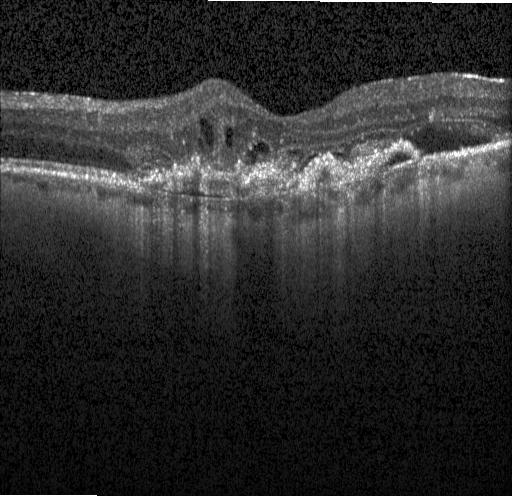
Macular scan, OCT B-scan, SD-OCT, instrument: Heidelberg Spectralis
Diagnosis: a choroidal neovascular membrane.